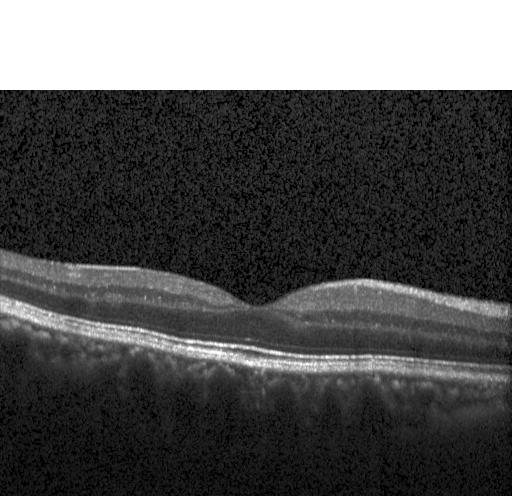

Retinal OCT cross-section showing no evidence of choroidal neovascularization, diabetic macular edema, or drusen.